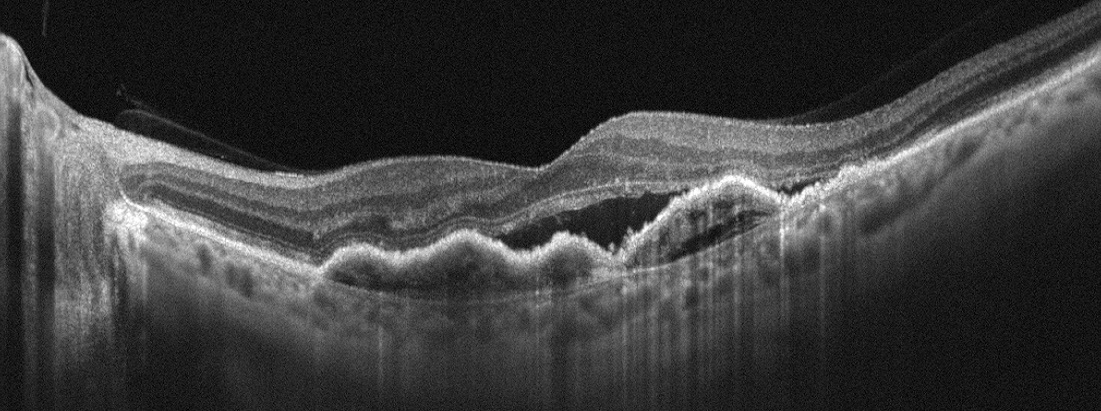 Fovea-centered · optical coherence tomography B-scan · instrument: Optovue Avanti RTVue XR
Macular OCT: age-related macular degeneration.